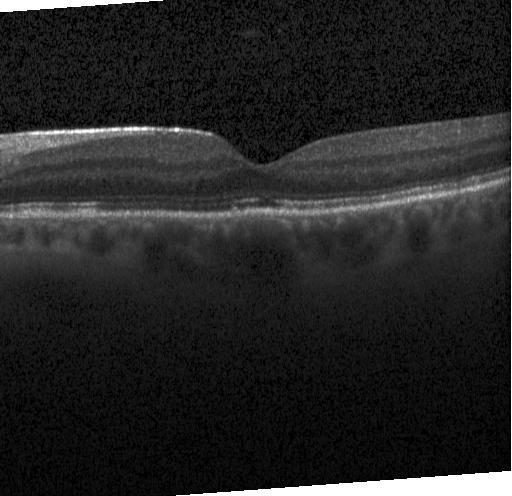
Retinal OCT cross-section
Macular OCT: neither choroidal neovascularization, diabetic macular edema, nor drusen.